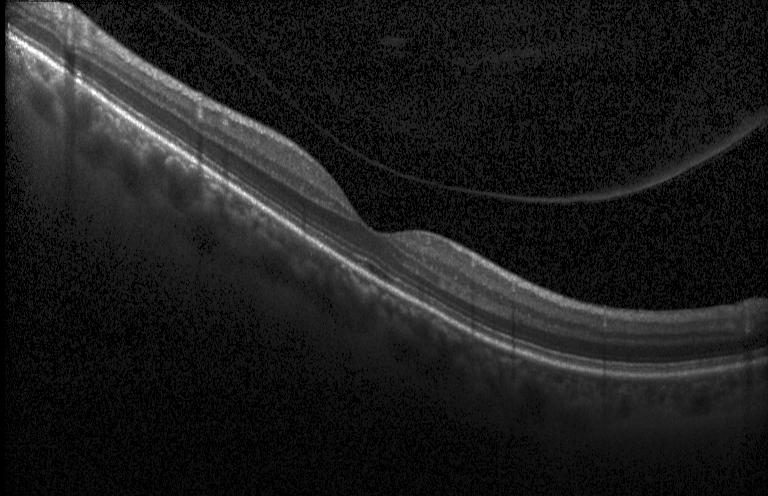

Diagnosis: no choroidal neovascularization, no diabetic macular edema, and no drusen.